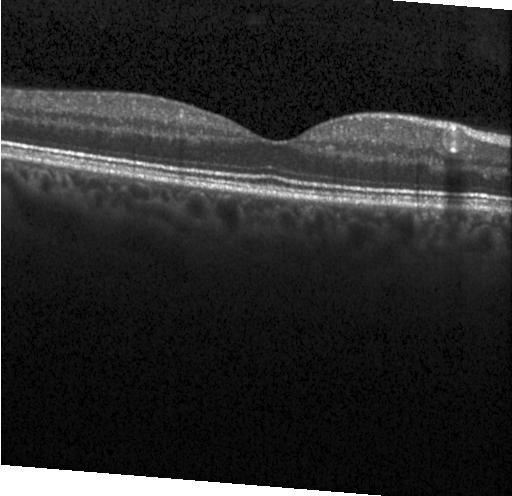

Centered on the fovea. Instrument: Heidelberg Spectralis. Spectral-domain OCT. Optical coherence tomography scan
Impression: neither choroidal neovascularization, diabetic macular edema, nor drusen.